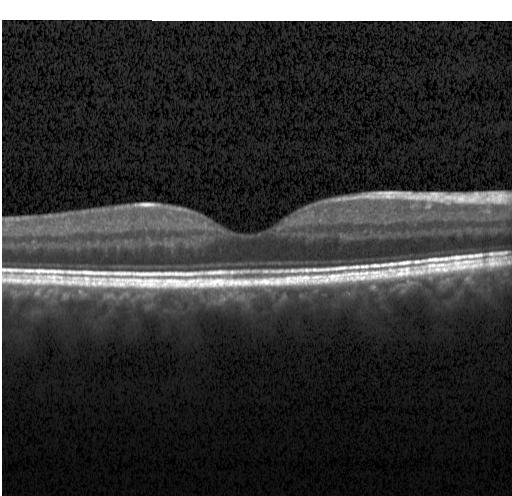 OCT line scan.
The scan shows no choroidal neovascularization, diabetic macular edema, or drusen.